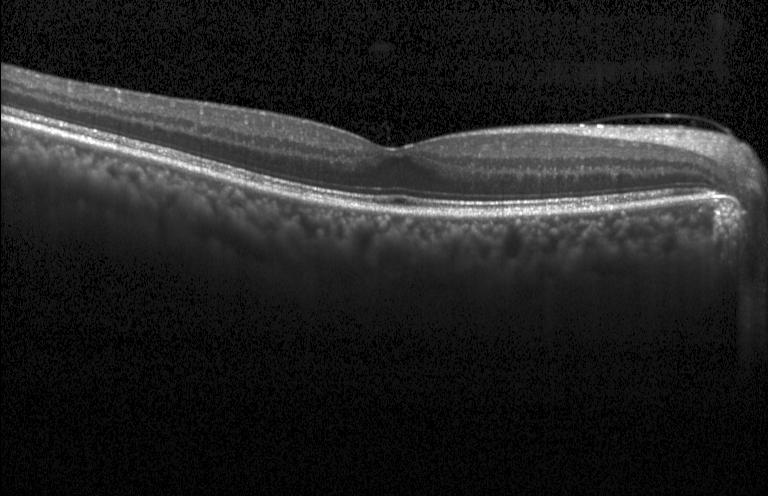

Retinal OCT cross-section — Impression: no evidence of choroidal neovascularization, diabetic macular edema, or drusen.